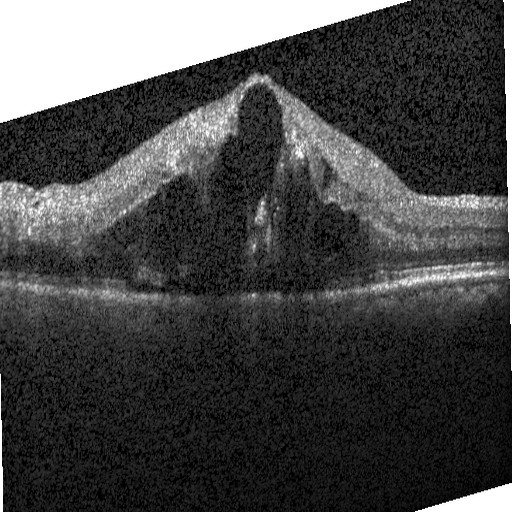 Heidelberg Spectralis. Spectral-domain OCT. Through the macula. Retinal OCT cross-section — Assessment: DME.